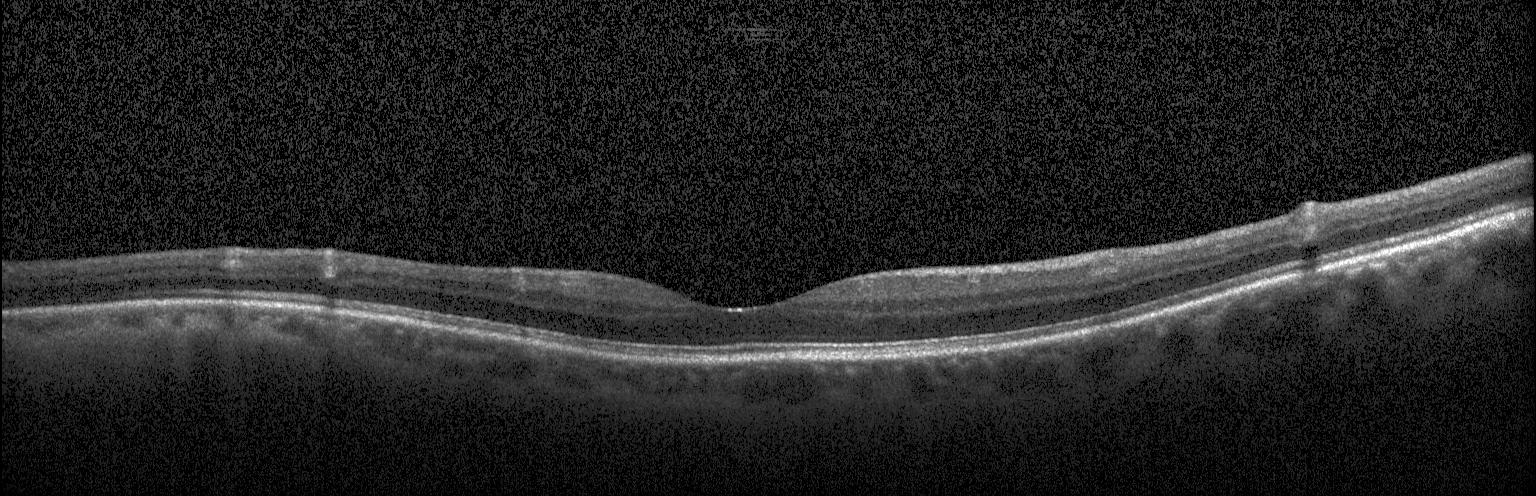

Spectral-domain optical coherence tomography; fovea-centered; OCT B-scan; acquired on a Heidelberg Spectralis.
The scan shows neither CNV, DME, nor drusen.